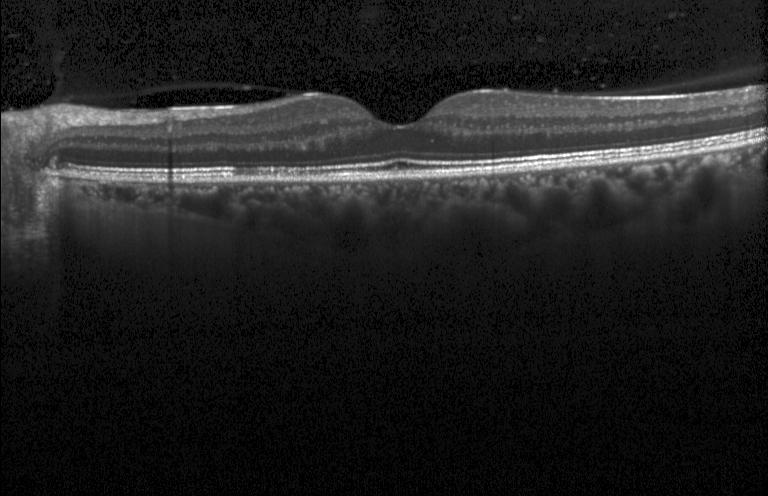
OCT B-scan — Finding: neither CNV, DME, nor drusen.